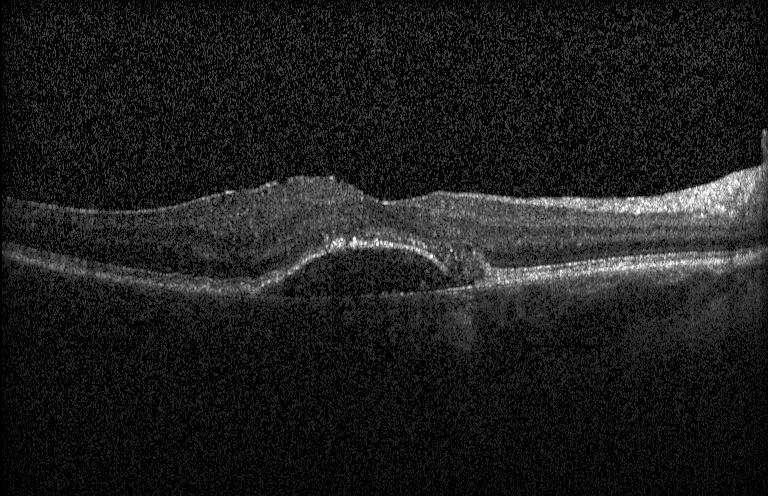
OCT B-scan.
OCT finding: choroidal neovascularization (CNV).